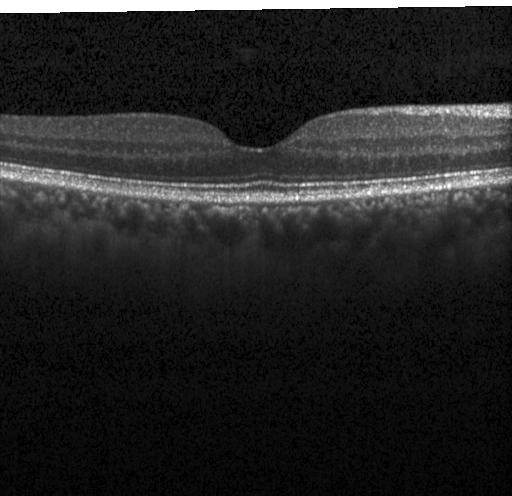

Macular OCT demonstrating no CNV, DME, or drusen.